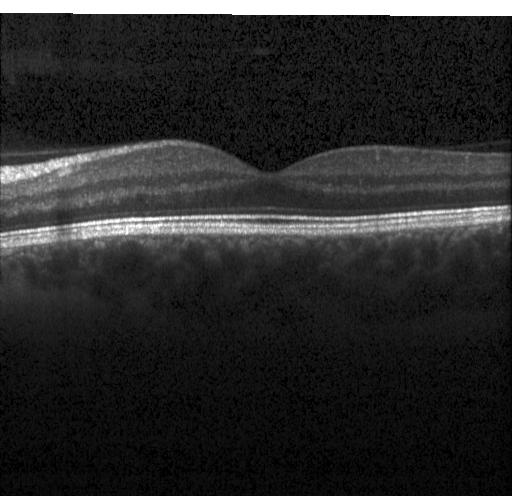

OCT B-scan · Heidelberg Spectralis OCT system · spectral-domain optical coherence tomography · centered on the fovea.
Impression: neither choroidal neovascularization, diabetic macular edema, nor drusen.